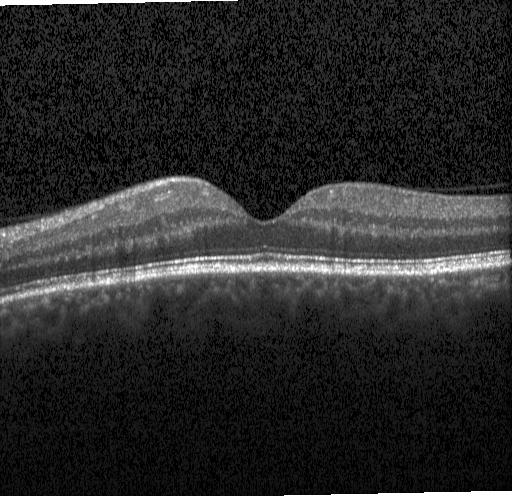

Dx: no evidence of CNV, DME, or drusen.